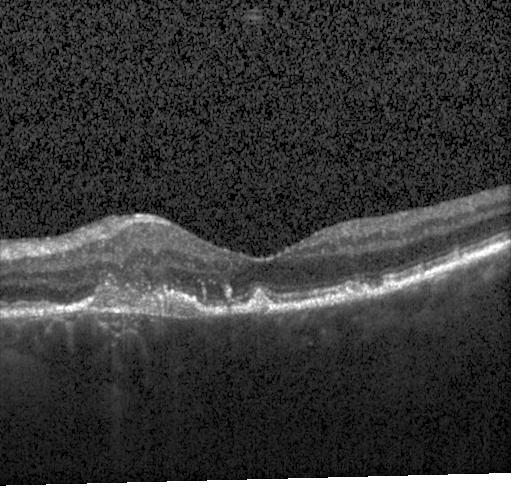

Macular scan, retinal OCT cross-section, spectral-domain optical coherence tomography.
Diagnosis: a choroidal neovascular membrane.